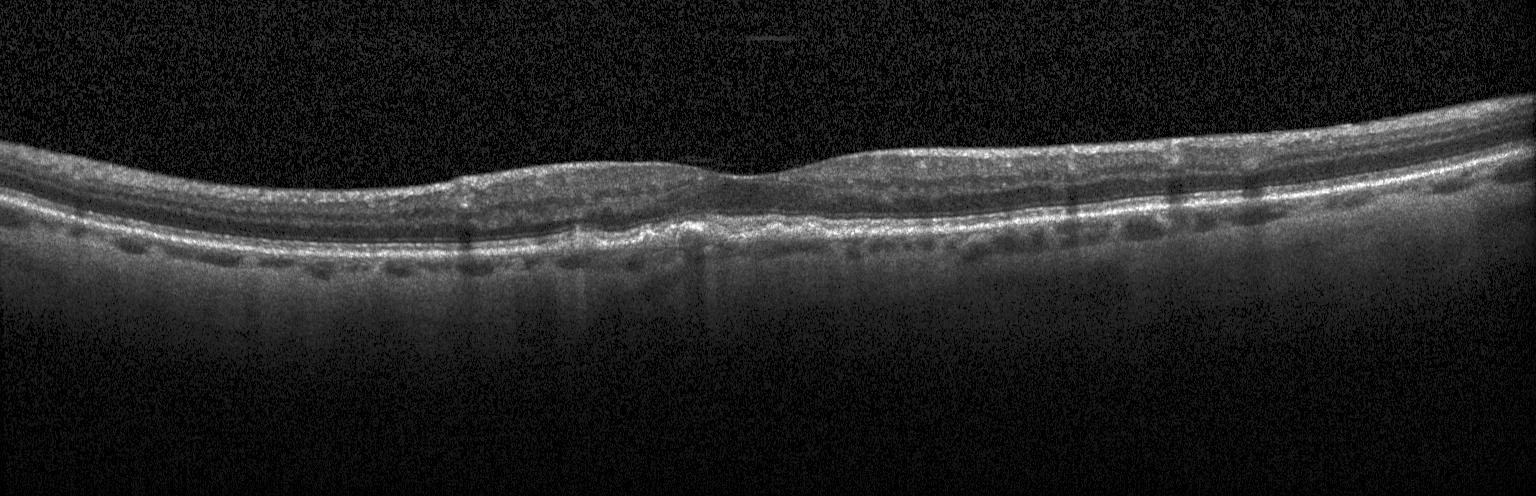
OCT finding: sub-RPE drusenoid deposits.